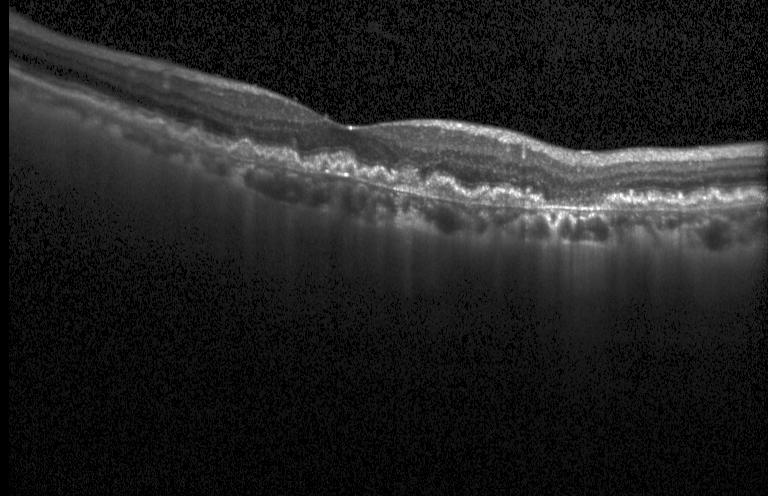 Dx: choroidal neovascularization (CNV).